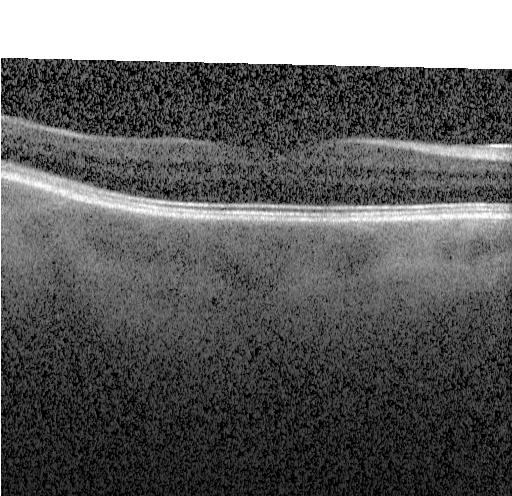

The scan shows no evidence of choroidal neovascularization, diabetic macular edema, or drusen.